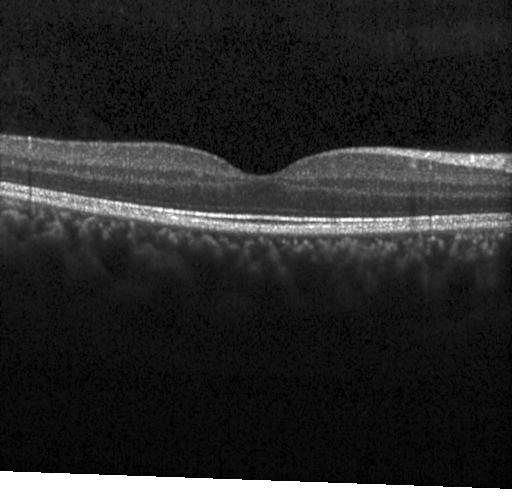
Finding: no evidence of CNV, DME, or drusen.